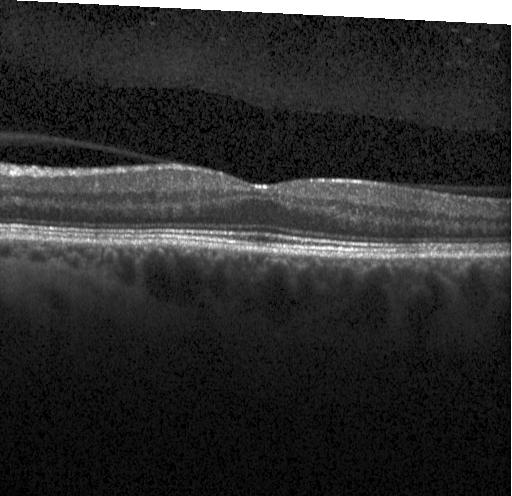

Impression: no choroidal neovascularization, no diabetic macular edema, and no drusen.